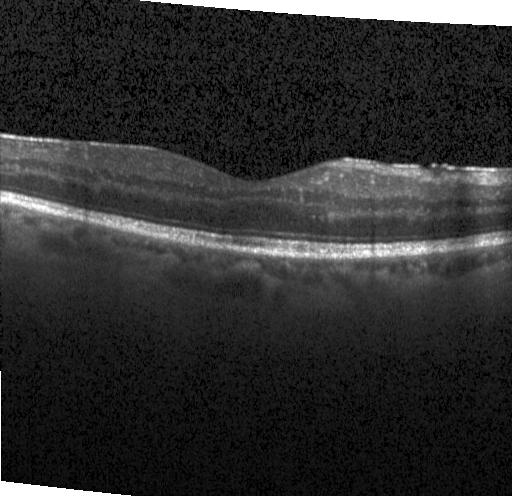

Retinal OCT cross-section · spectral-domain OCT — Finding: neither CNV, DME, nor drusen.